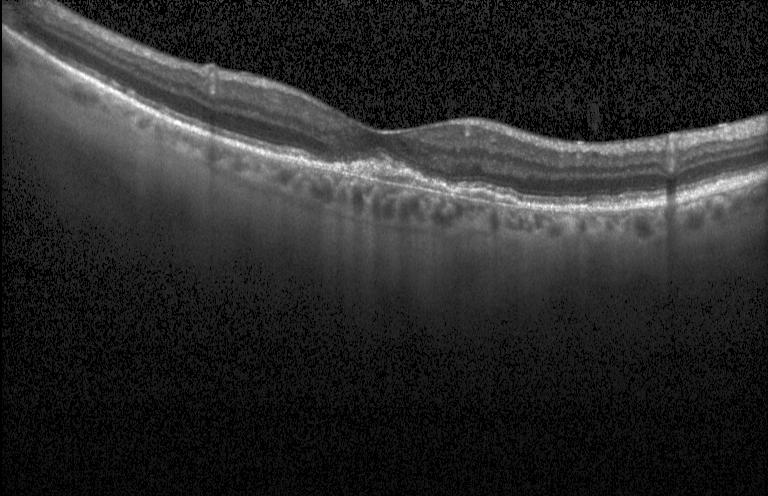

Retinal OCT cross-section; spectral-domain OCT; through the macula; acquired on a Heidelberg Spectralis
This B-scan demonstrates a choroidal neovascular membrane.